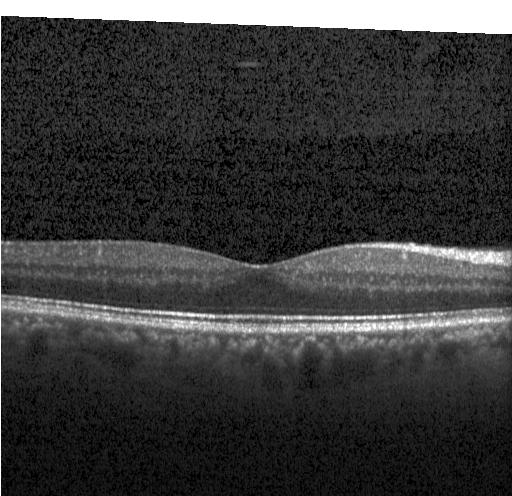
Dx: no evidence of choroidal neovascularization, diabetic macular edema, or drusen.